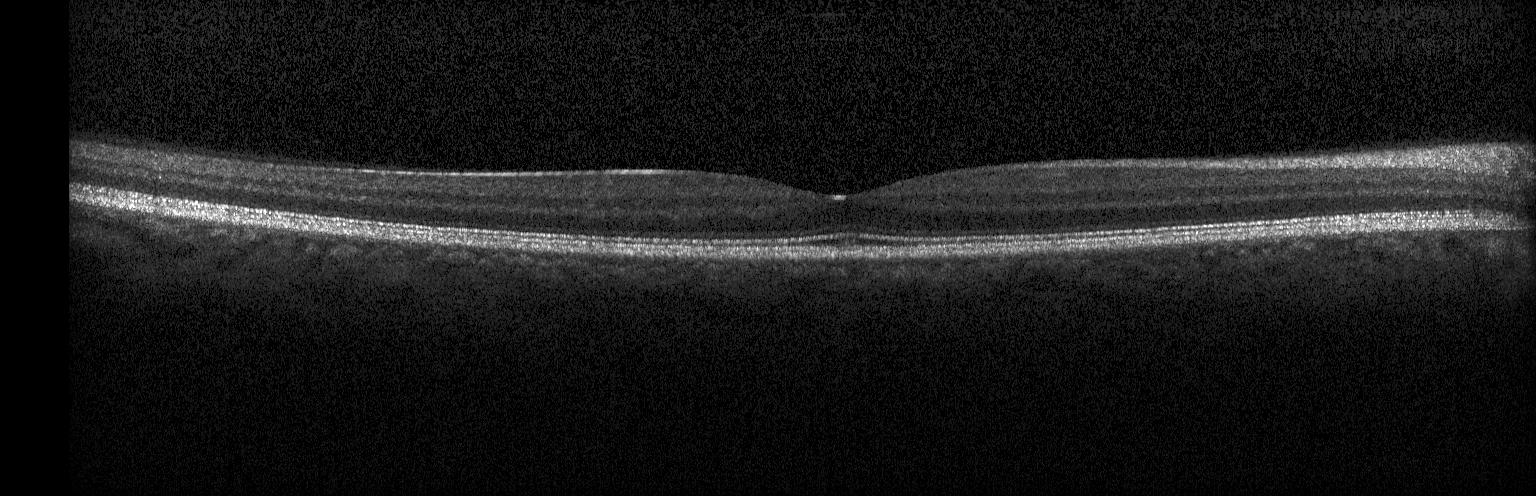
Diagnosis: no evidence of choroidal neovascularization, diabetic macular edema, or drusen.